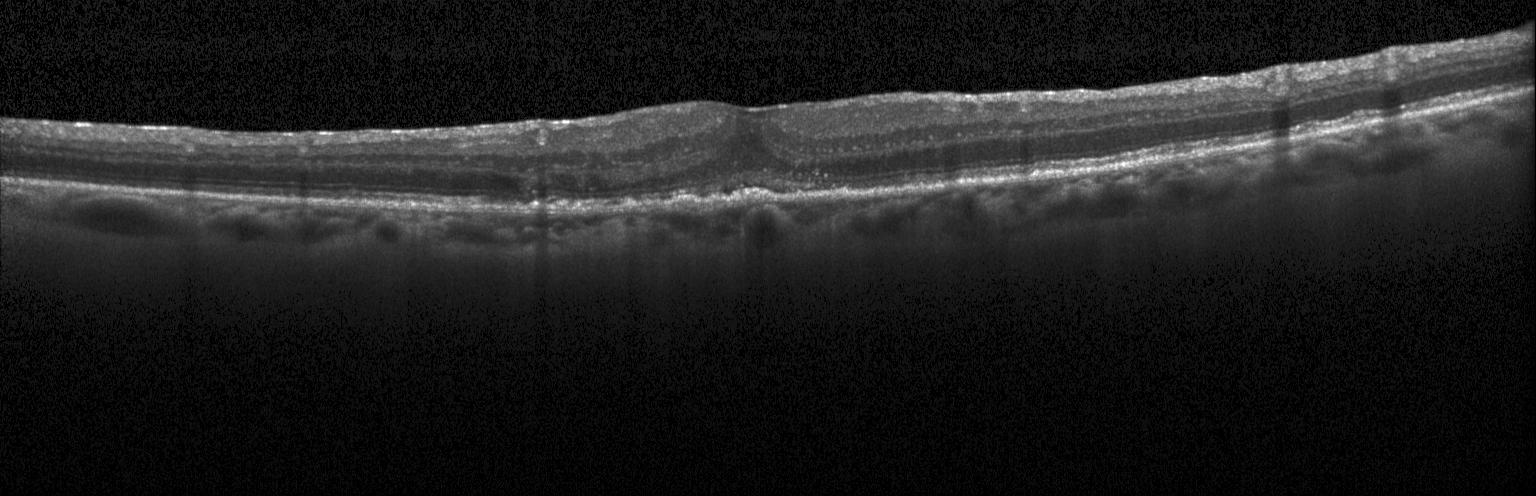
Heidelberg Spectralis OCT system; OCT B-scan
Impression: a choroidal neovascular membrane.